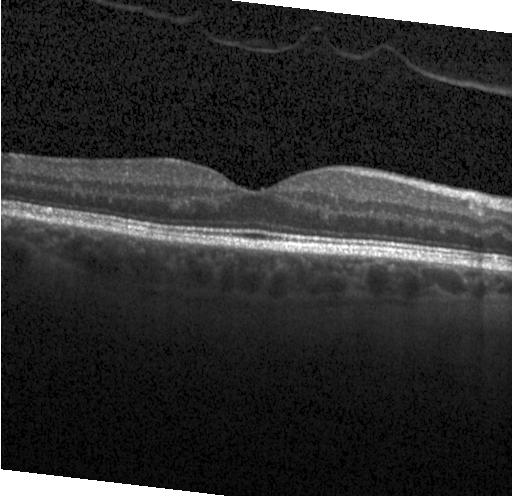

Optical coherence tomography B-scan — No CNV, no DME, and no drusen.